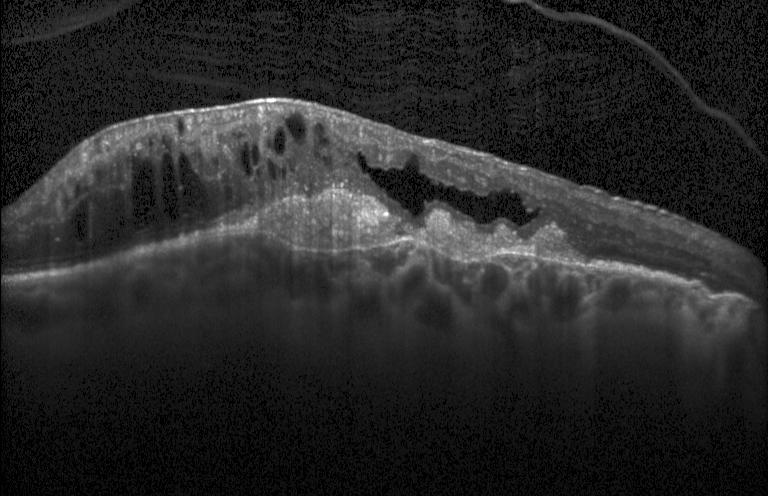 OCT finding: a choroidal neovascular membrane.